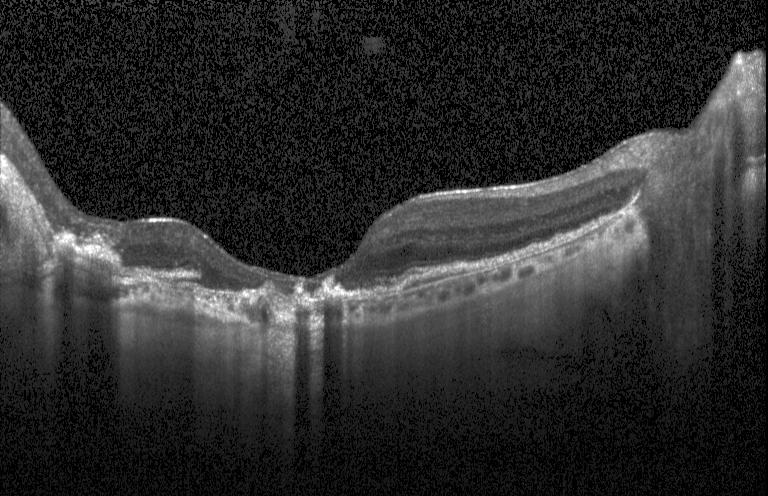

Optical coherence tomography scan. Finding: CNV.